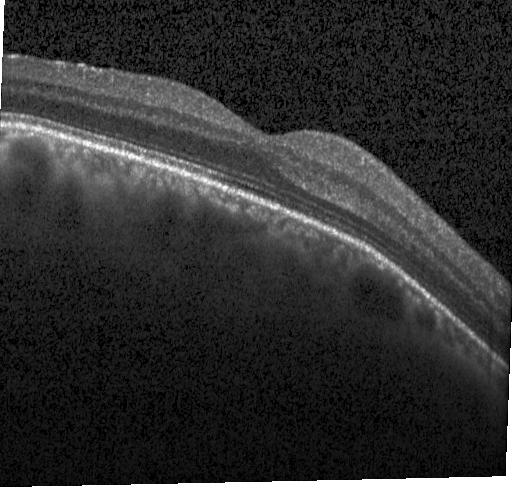

Retinal OCT cross-section; SD-OCT.
Dx: no CNV, DME, or drusen.